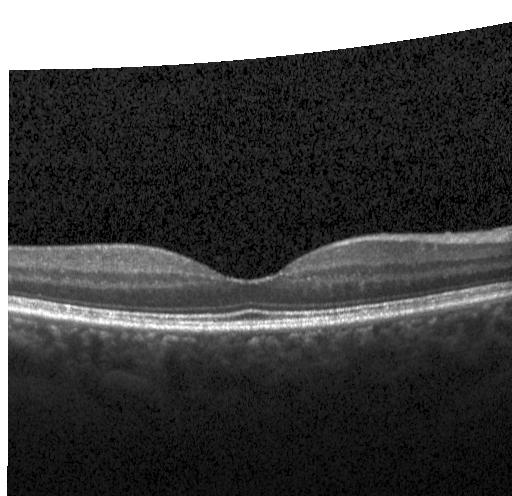

Optical coherence tomography B-scan — Finding: no choroidal neovascularization, no diabetic macular edema, and no drusen.